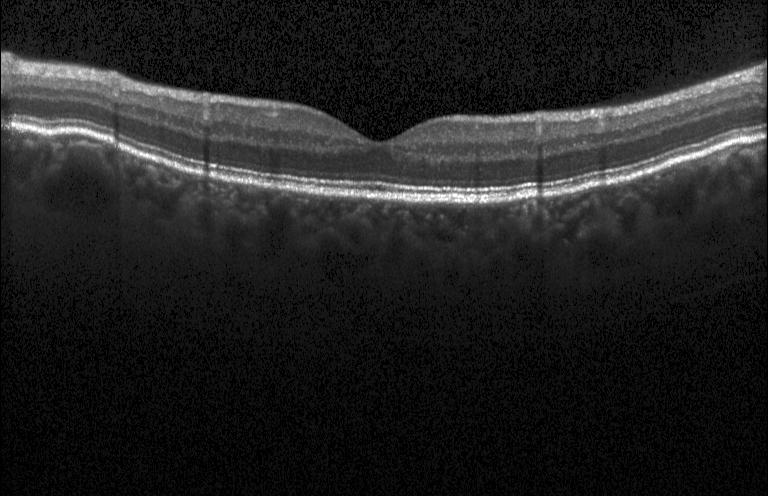

The scan shows no CNV, no DME, and no drusen.